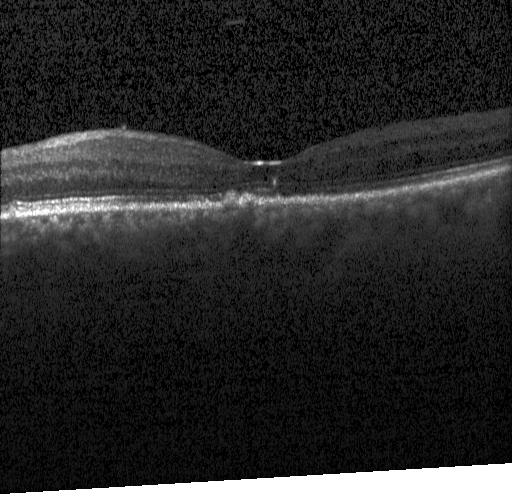 SD-OCT · retinal OCT cross-section
The scan shows sub-RPE drusenoid deposits.